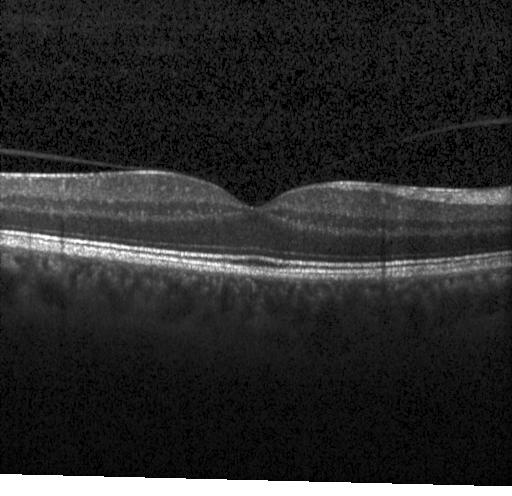
SD-OCT, fovea-centered, OCT line scan. No CNV, DME, or drusen.